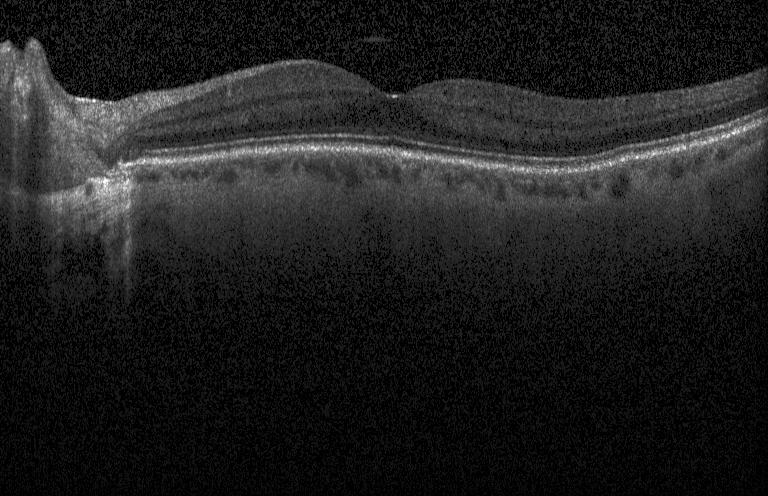 Retinal OCT cross-section; instrument: Heidelberg Spectralis; spectral-domain OCT.
Impression: no choroidal neovascularization, no diabetic macular edema, and no drusen.